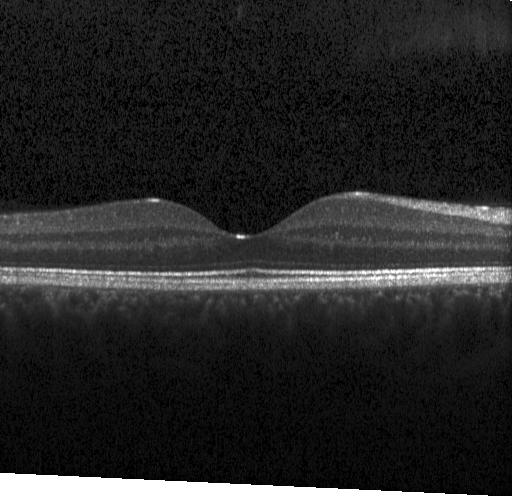 Instrument: Heidelberg Spectralis, optical coherence tomography scan
Finding: no CNV, DME, or drusen.